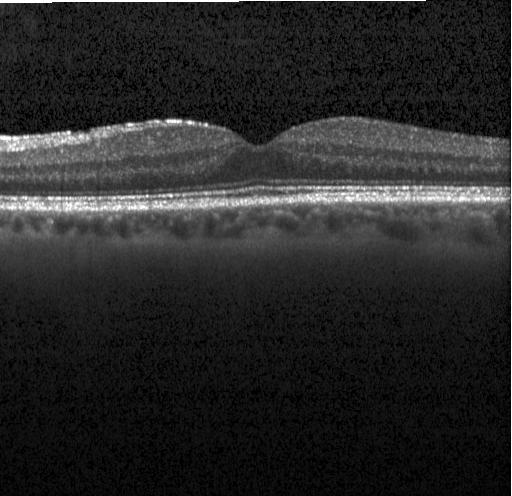

SD-OCT. Heidelberg Spectralis OCT system. Retinal OCT cross-section. Centered on the fovea. Finding: neither choroidal neovascularization, diabetic macular edema, nor drusen.